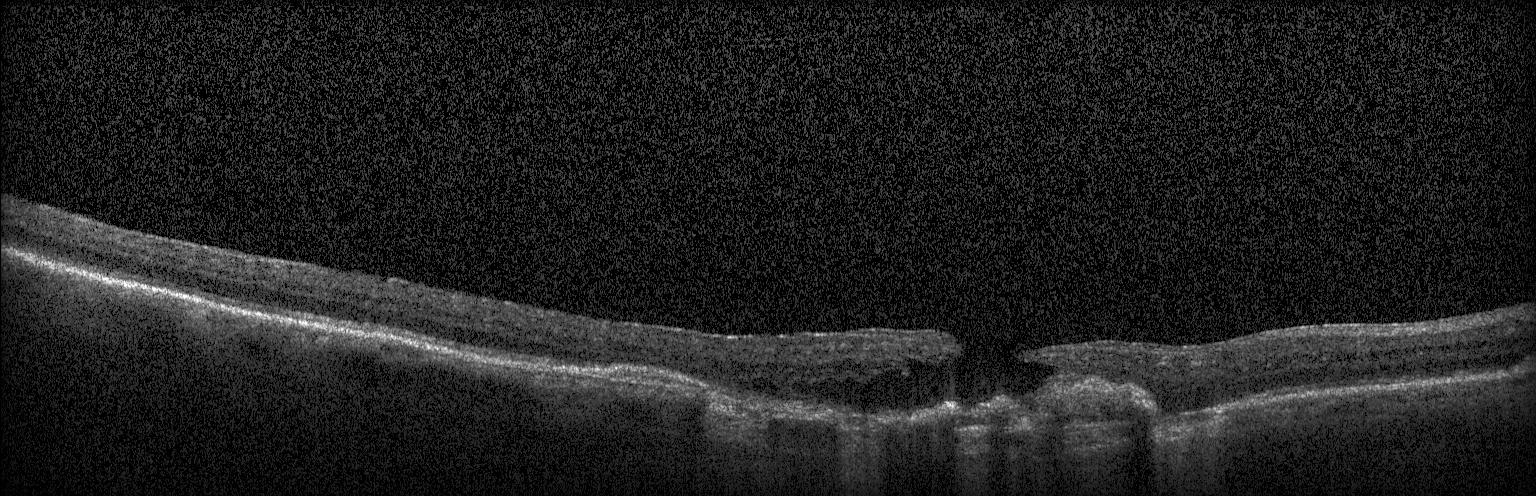
Retinal OCT B-scan.
Assessment: CNV.